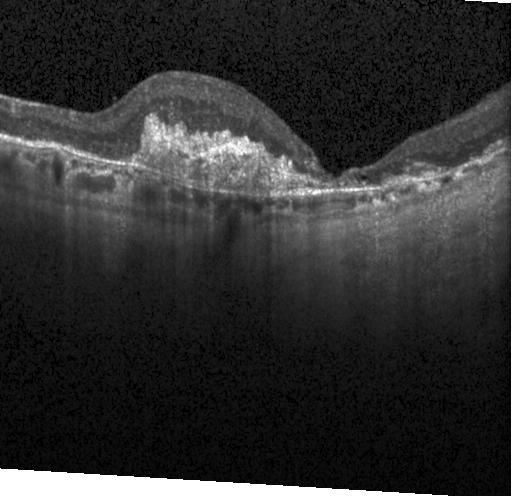
Spectral-domain OCT. Through the macula. Instrument: Heidelberg Spectralis. OCT B-scan — Diagnosis: a choroidal neovascular membrane.